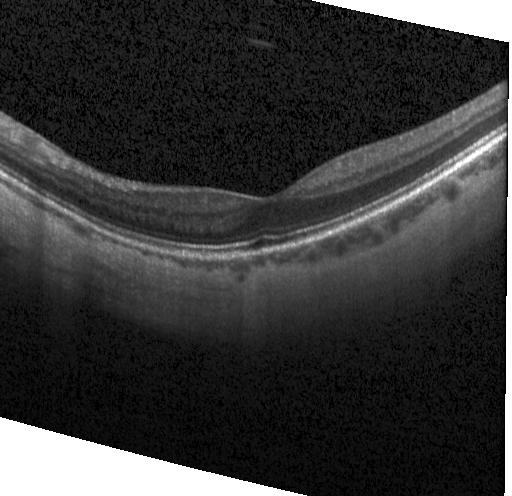 Optical coherence tomography B-scan
Impression: neither choroidal neovascularization, diabetic macular edema, nor drusen.